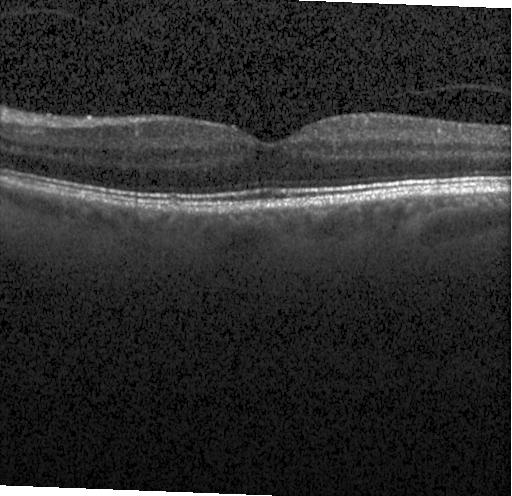
OCT B-scan, spectral-domain optical coherence tomography.
Diagnosis: no CNV, DME, or drusen.